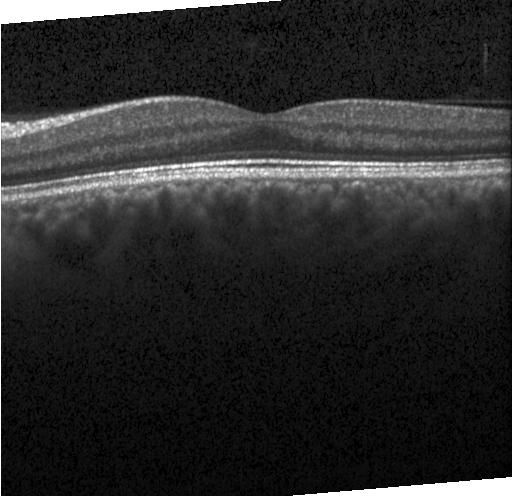
Optical coherence tomography B-scan.
Finding: no choroidal neovascularization, diabetic macular edema, or drusen.